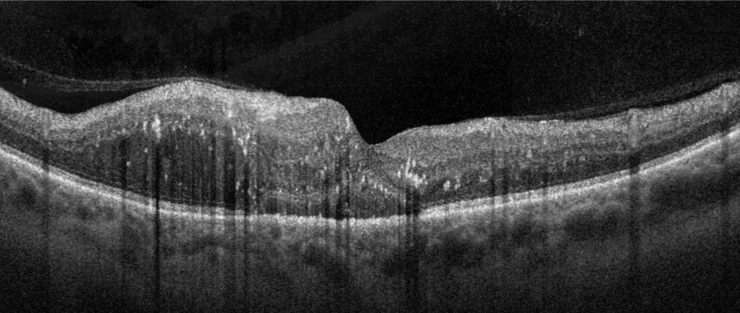 Retinal OCT B-scan
Diagnosis: DME.